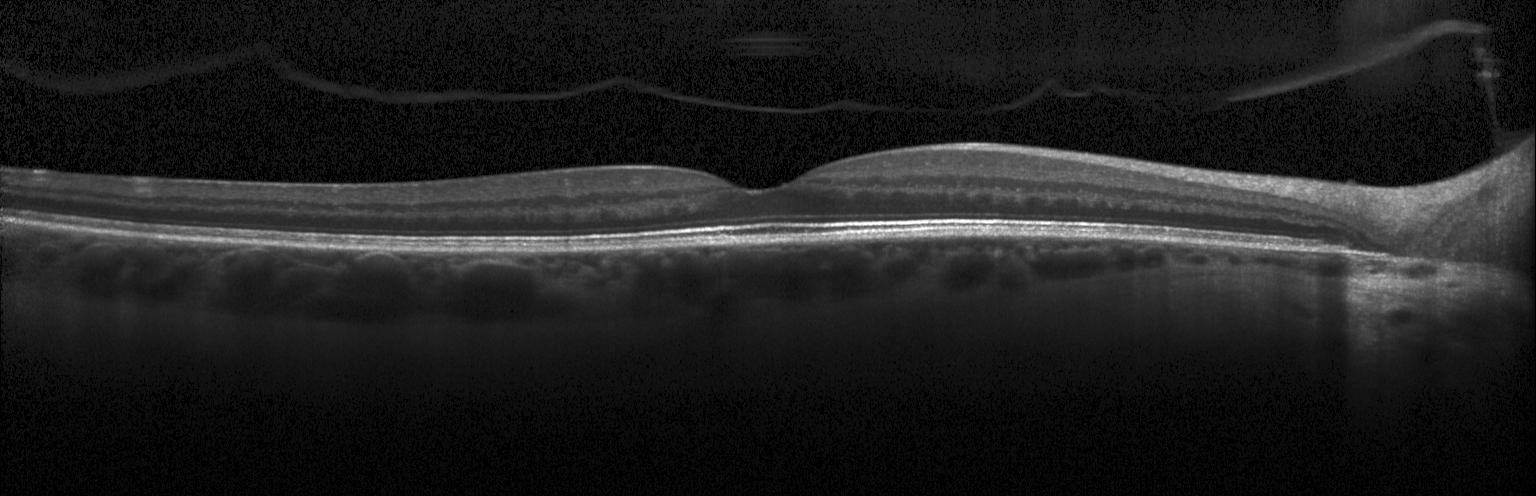
Spectral-domain optical coherence tomography. Horizontal scan through the fovea. Heidelberg Spectralis. OCT B-scan.
Dx: no evidence of choroidal neovascularization, diabetic macular edema, or drusen.